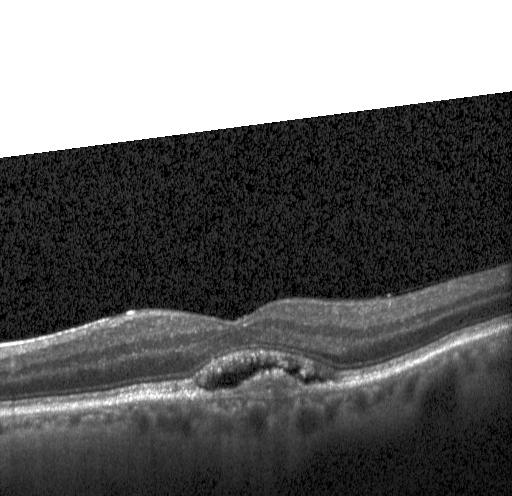
Assessment: a choroidal neovascular membrane.